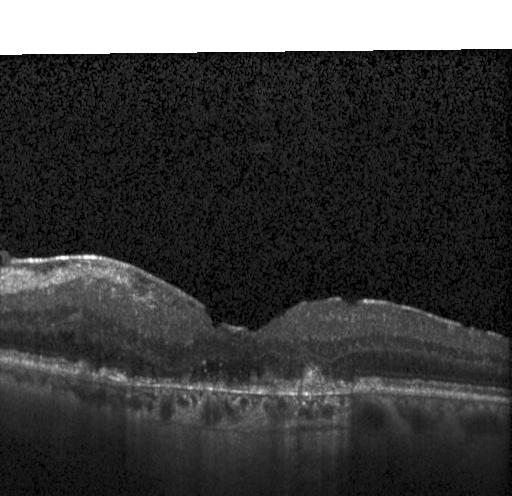

Instrument: Heidelberg Spectralis. OCT B-scan
Macular OCT: a choroidal neovascular membrane.